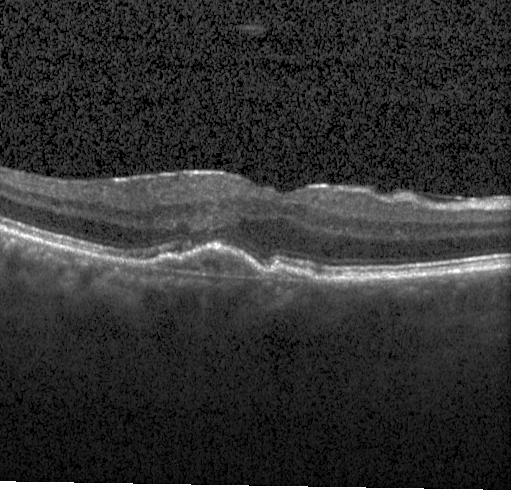
Instrument: Heidelberg Spectralis · retinal OCT B-scan · SD-OCT. Diagnosis: choroidal neovascularization (CNV).